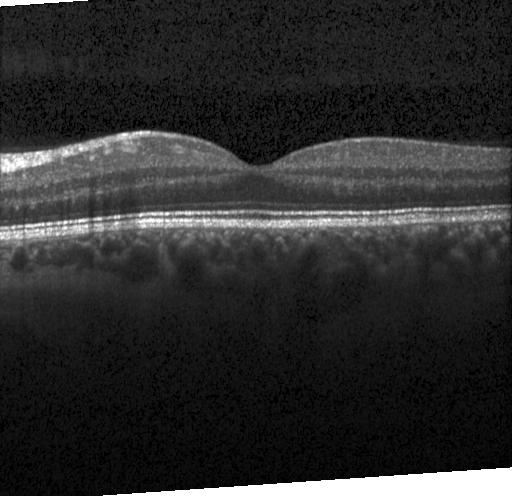
The scan shows no choroidal neovascularization, diabetic macular edema, or drusen.